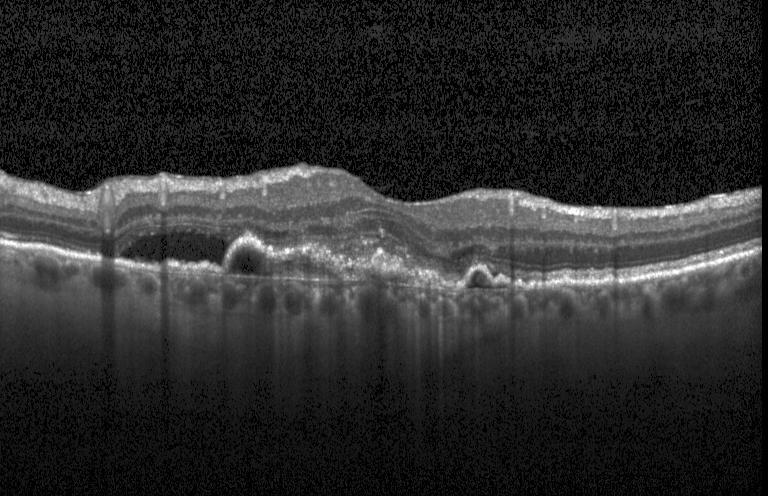 Acquired on a Heidelberg Spectralis · centered on the fovea · OCT B-scan — Diagnosis: a choroidal neovascular membrane.